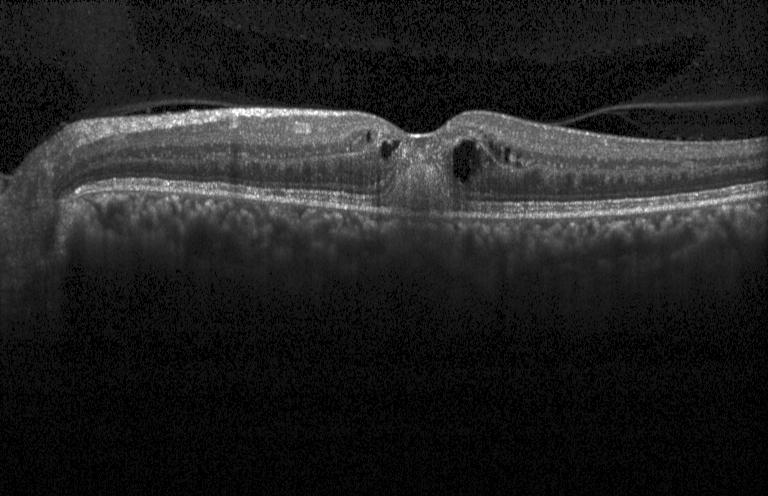

This B-scan demonstrates a choroidal neovascular membrane.